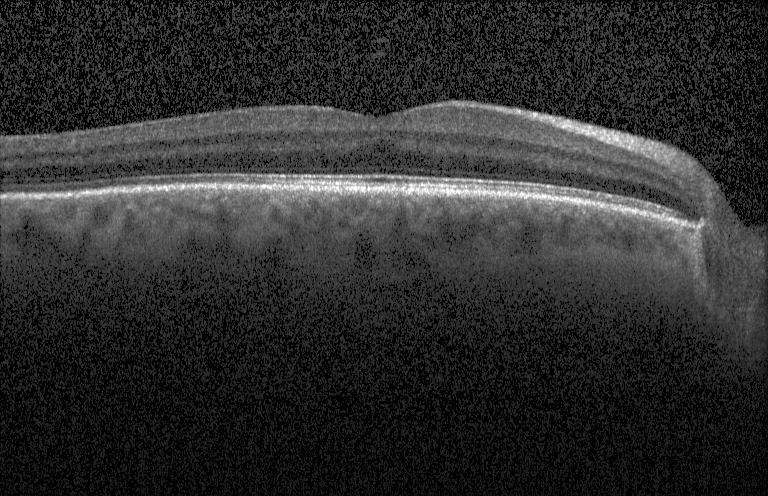 Retinal OCT B-scan · spectral-domain optical coherence tomography · fovea-centered · Heidelberg Spectralis OCT system
Diagnosis: no CNV, DME, or drusen.